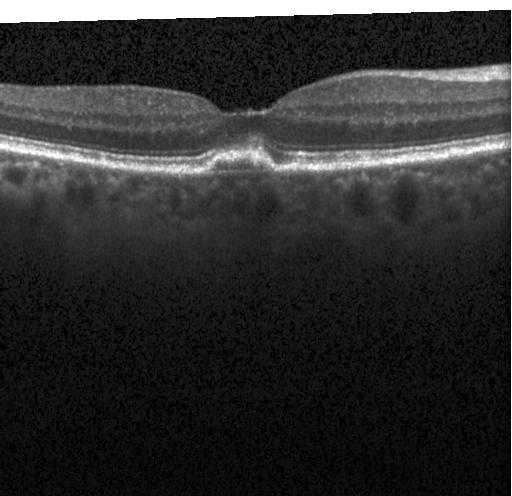
Macular scan · optical coherence tomography B-scan. Impression: choroidal neovascularization.